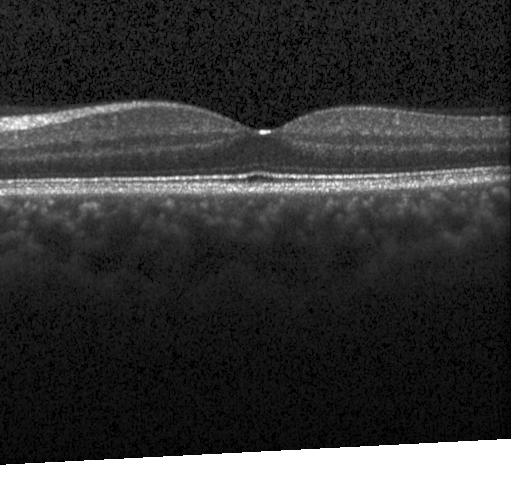 Dx: neither choroidal neovascularization, diabetic macular edema, nor drusen.